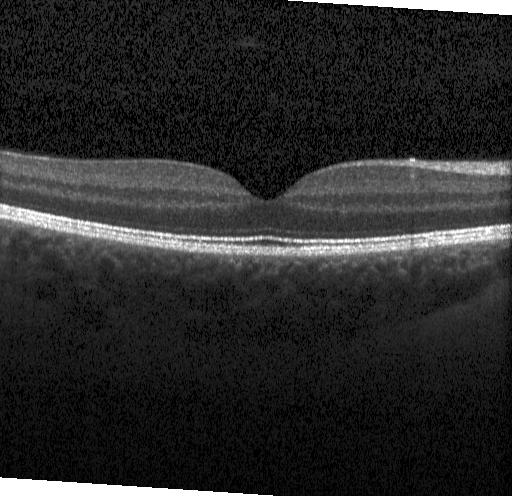
Optical coherence tomography B-scan · centered on the fovea · spectral-domain OCT · Heidelberg Spectralis
Diagnosis: no evidence of CNV, DME, or drusen.